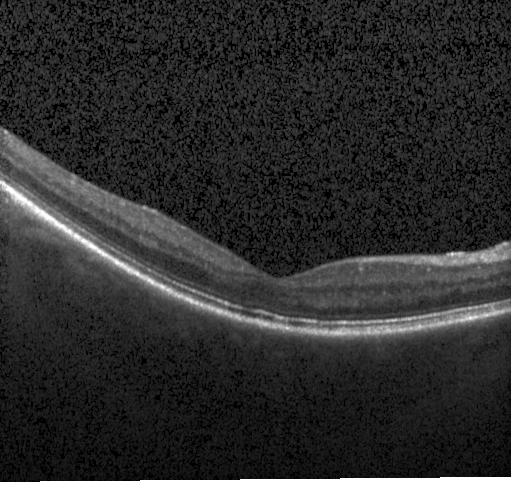

Macular scan; SD-OCT; OCT line scan; Heidelberg Spectralis OCT system — Finding: no evidence of choroidal neovascularization, diabetic macular edema, or drusen.